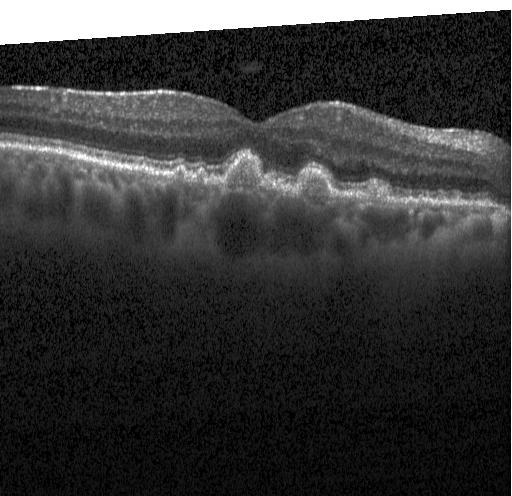

Optical coherence tomography B-scan, through the macula, spectral-domain OCT, acquired on a Heidelberg Spectralis. This B-scan demonstrates drusen.